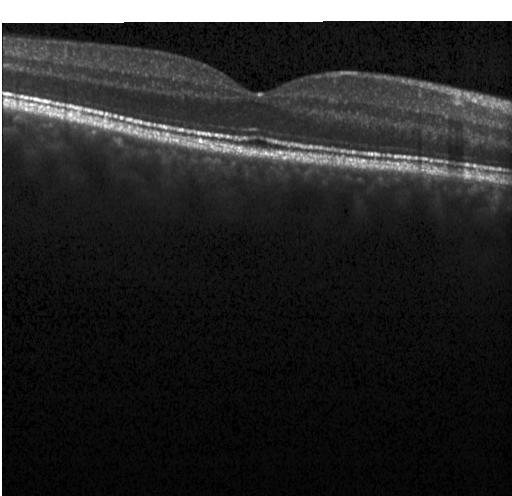 Diagnosis: no evidence of CNV, DME, or drusen.